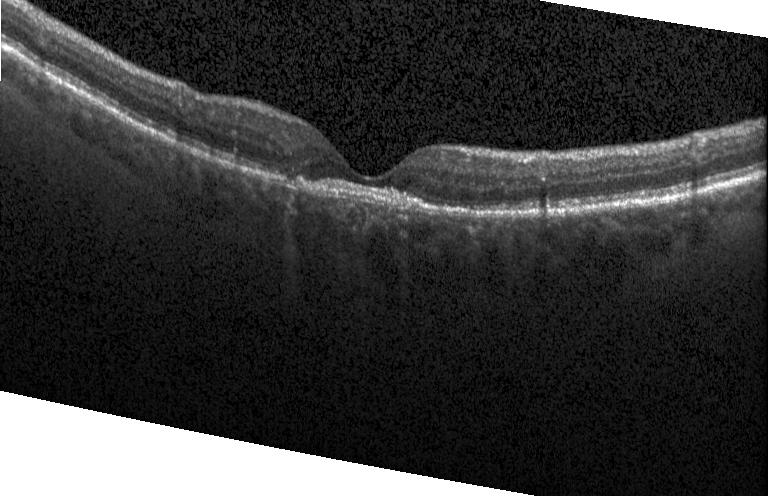 Macular scan · SD-OCT · instrument: Heidelberg Spectralis · retinal OCT cross-section. Finding: CNV.